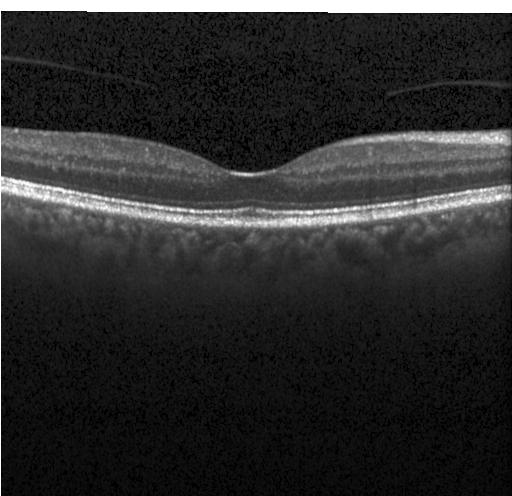

Diagnosis: neither CNV, DME, nor drusen.